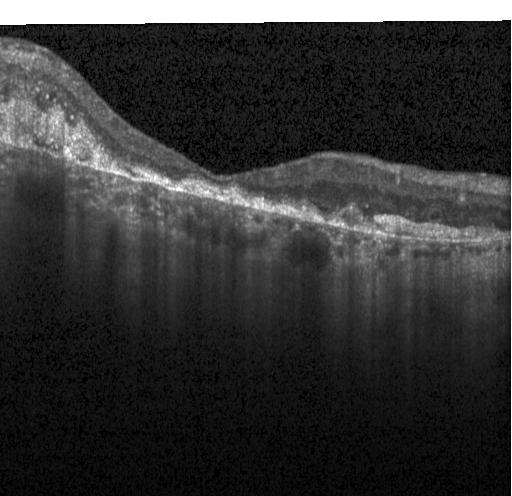
OCT line scan. Impression: choroidal neovascularization (CNV).